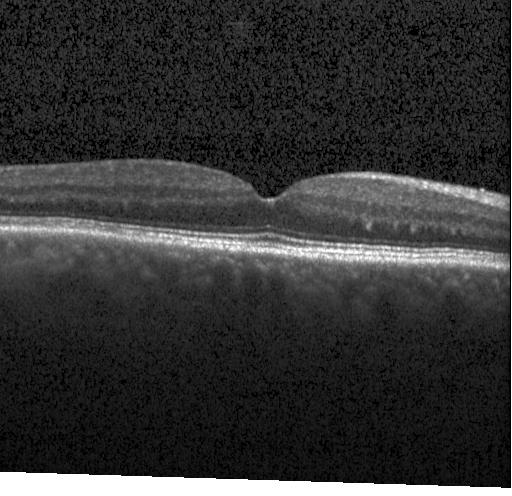 Finding: no choroidal neovascularization, no diabetic macular edema, and no drusen.